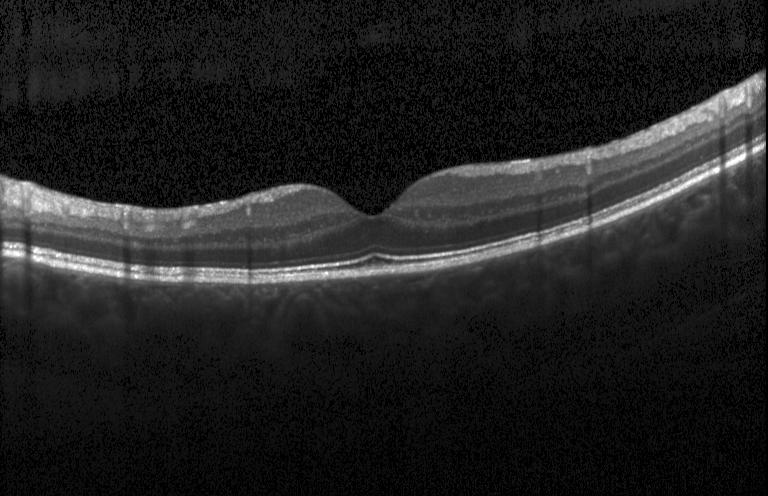
Macular OCT: no choroidal neovascularization, no diabetic macular edema, and no drusen.